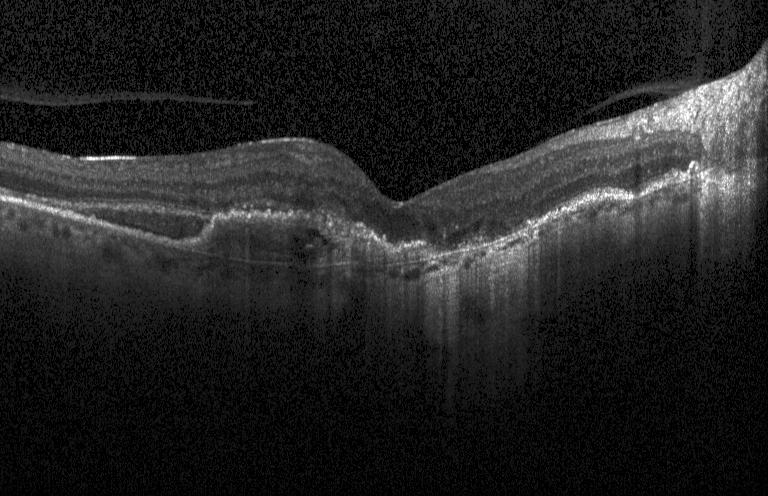

Impression: a choroidal neovascular membrane.